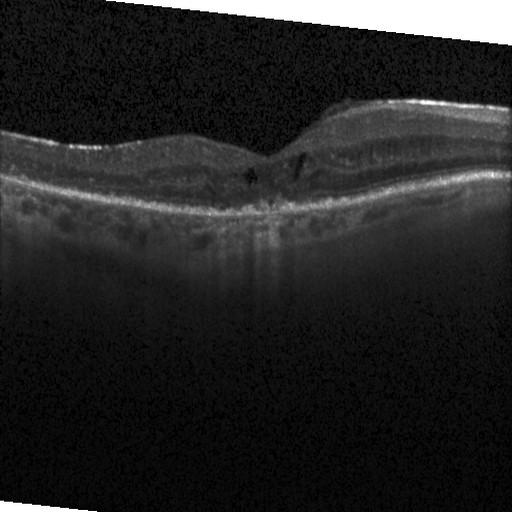

SD-OCT · optical coherence tomography B-scan.
Finding: DME.